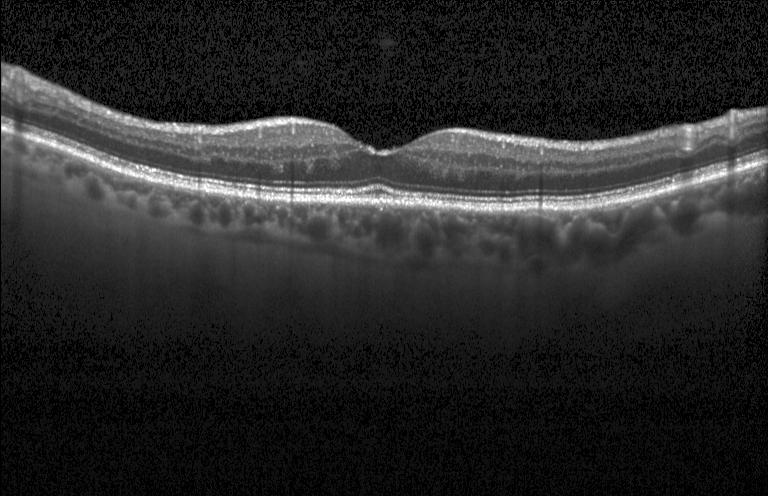
OCT line scan, spectral-domain optical coherence tomography. Assessment: no CNV, no DME, and no drusen.